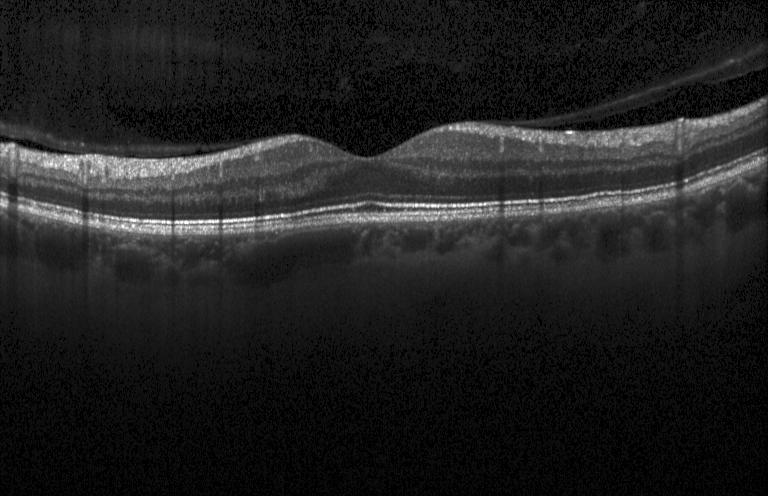 Heidelberg Spectralis. Optical coherence tomography B-scan — The scan shows no CNV, no DME, and no drusen.